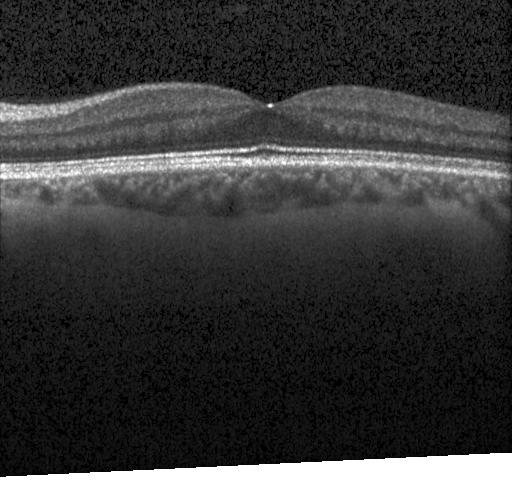

Retinal OCT B-scan — Impression: no evidence of CNV, DME, or drusen.